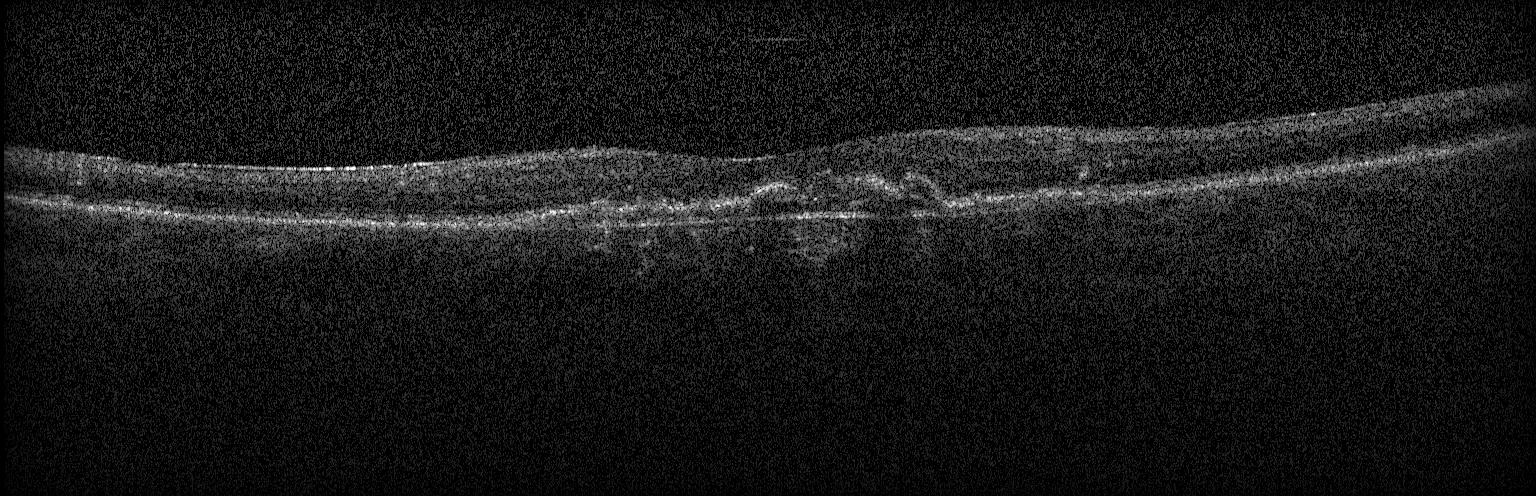
Spectral-domain optical coherence tomography. OCT line scan — This B-scan demonstrates a choroidal neovascular membrane.